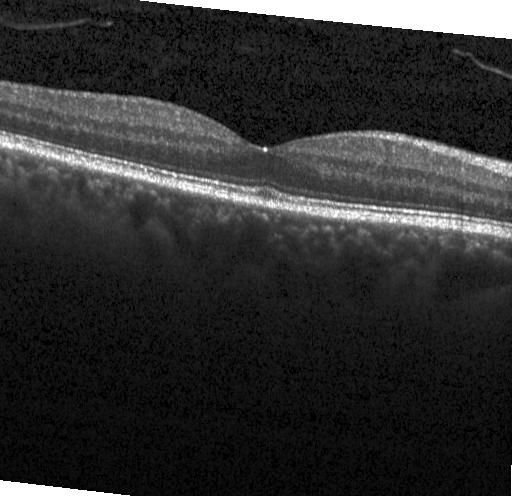 This B-scan demonstrates no evidence of choroidal neovascularization, diabetic macular edema, or drusen.